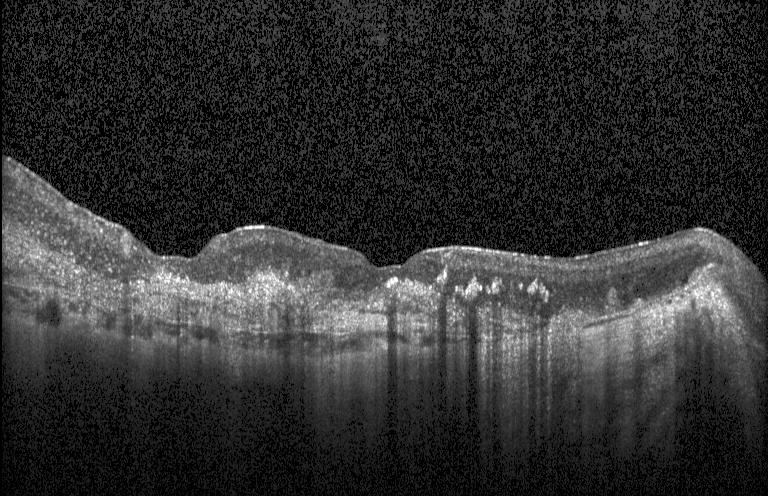
Retinal OCT cross-section. Heidelberg Spectralis. Fovea-centered
Diagnosis: choroidal neovascularization (CNV).